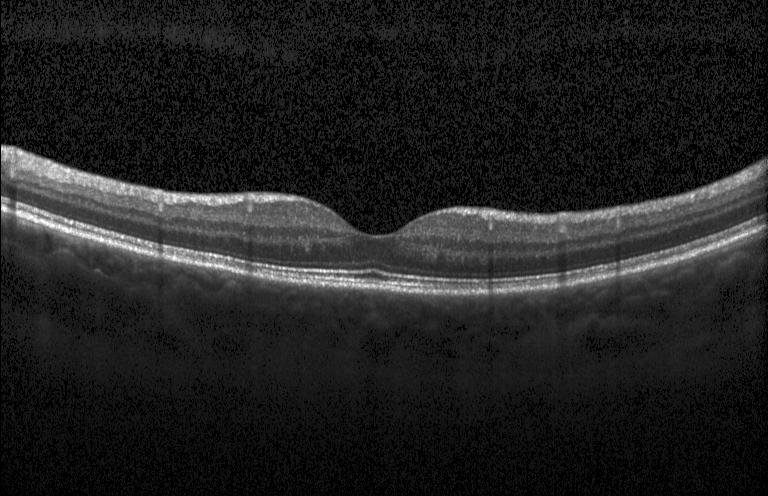
Spectral-domain optical coherence tomography. Retinal OCT B-scan.
OCT finding: no CNV, DME, or drusen.